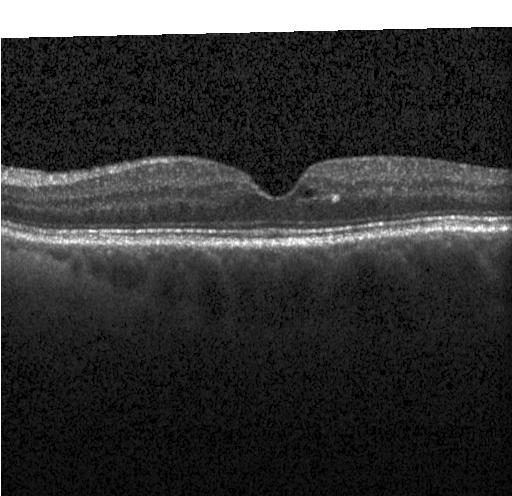 Acquired on a Heidelberg Spectralis; retinal OCT B-scan; spectral-domain optical coherence tomography; macular scan.
Dx: DME.